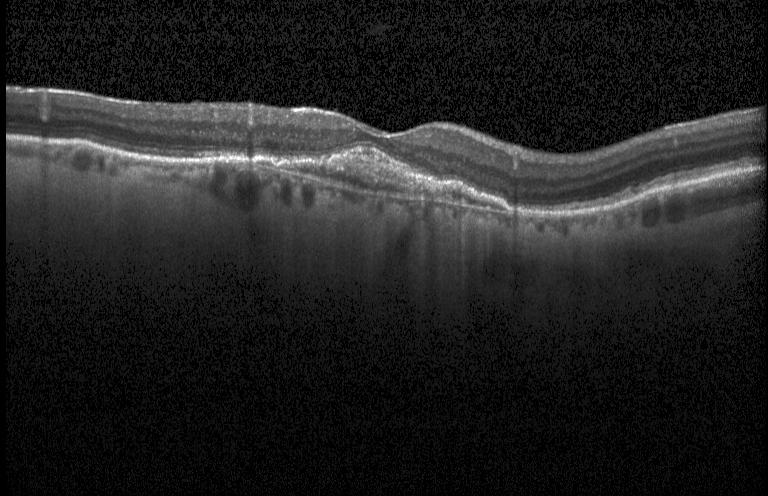

Optical coherence tomography scan — The scan shows a choroidal neovascular membrane.